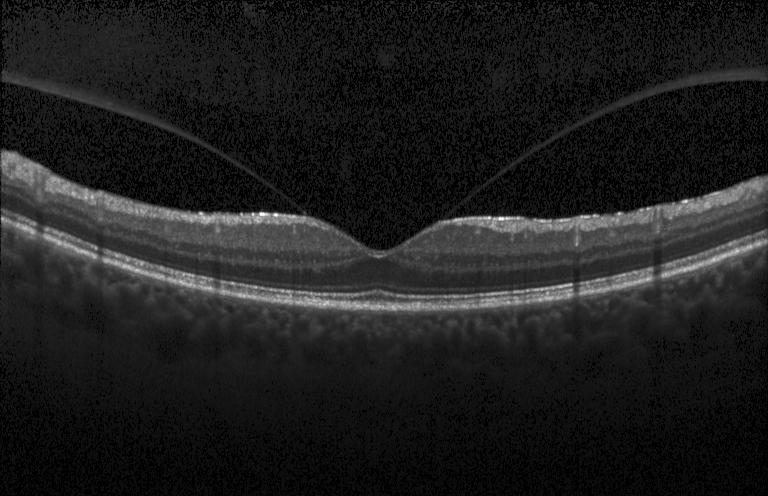
OCT line scan — No CNV, no DME, and no drusen.